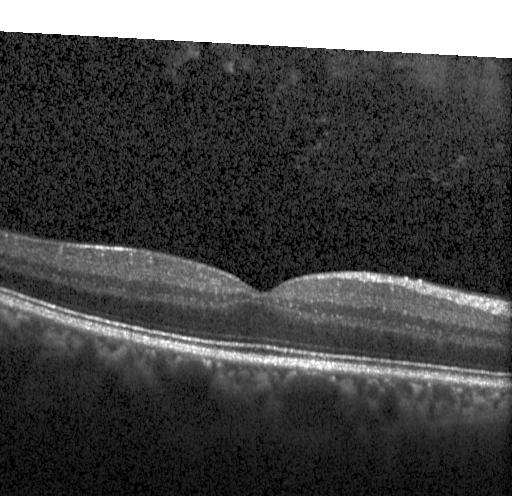

Macular scan · SD-OCT · OCT line scan
Dx: no choroidal neovascularization, diabetic macular edema, or drusen.